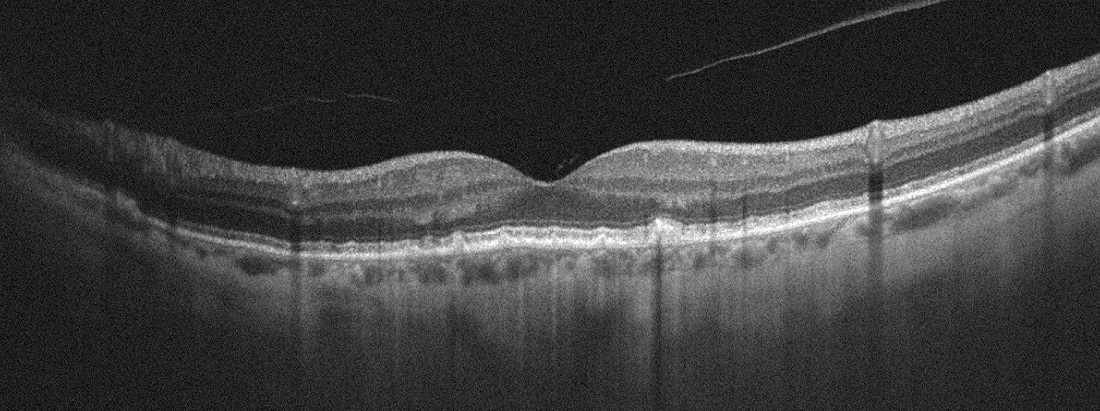 Acquired on an Optovue Avanti RTVue XR · retinal OCT cross-section. Dx: age-related macular degeneration (AMD).